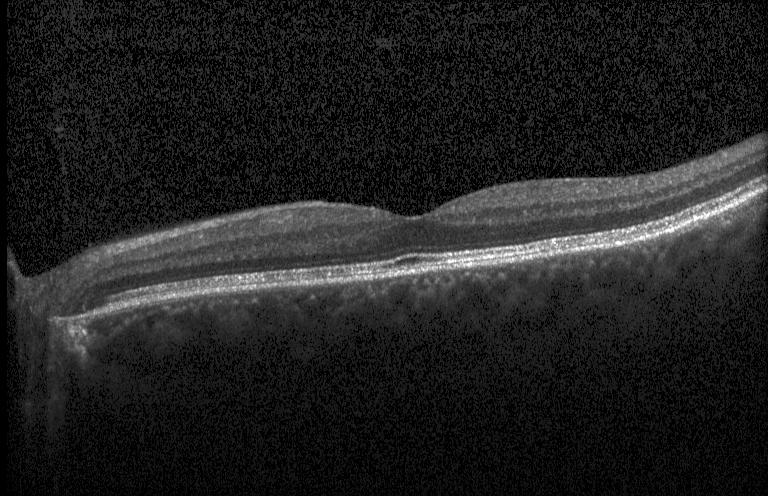
OCT line scan; centered on the fovea; spectral-domain OCT; acquired on a Heidelberg Spectralis.
Assessment: no choroidal neovascularization, diabetic macular edema, or drusen.